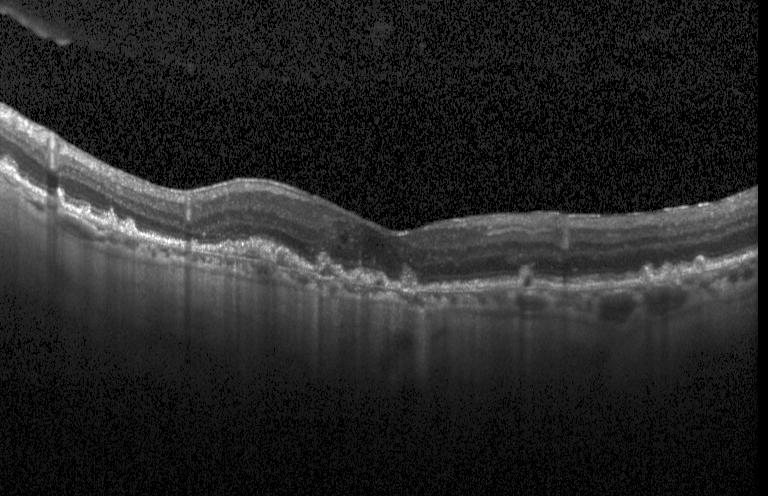 CNV.